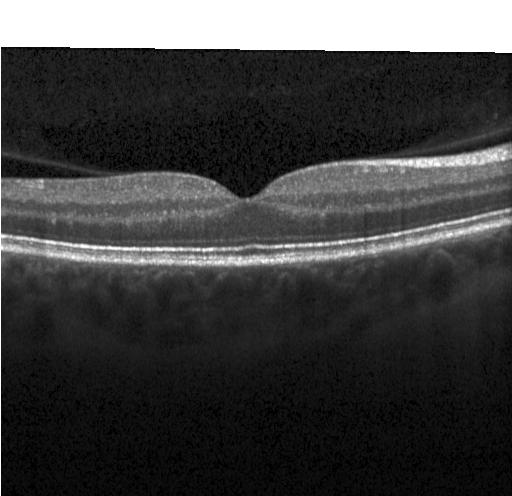
OCT line scan. Centered on the fovea.
Neither CNV, DME, nor drusen.